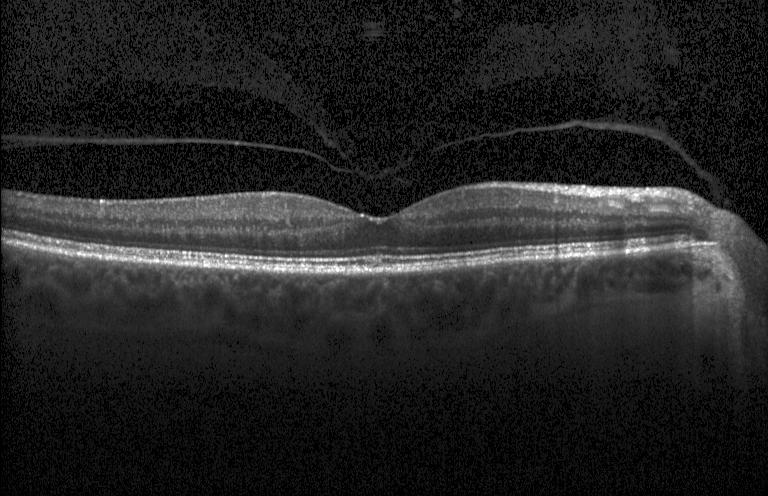

Finding: no evidence of CNV, DME, or drusen.